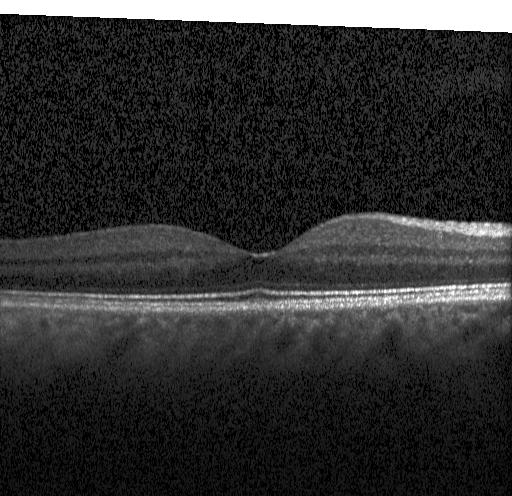
Spectral-domain optical coherence tomography, optical coherence tomography B-scan, instrument: Heidelberg Spectralis — Diagnosis: no evidence of choroidal neovascularization, diabetic macular edema, or drusen.